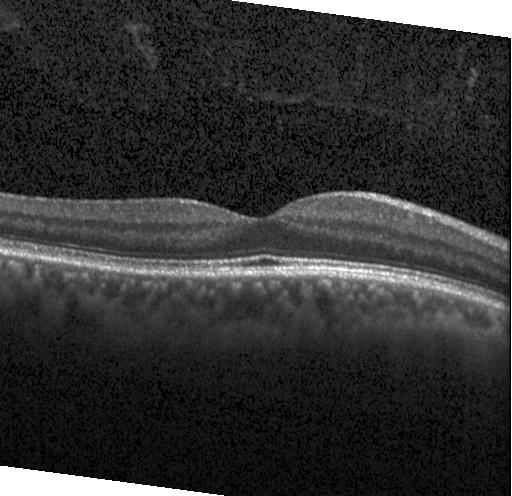 Spectral-domain OCT B-scan: no choroidal neovascularization, no diabetic macular edema, and no drusen.